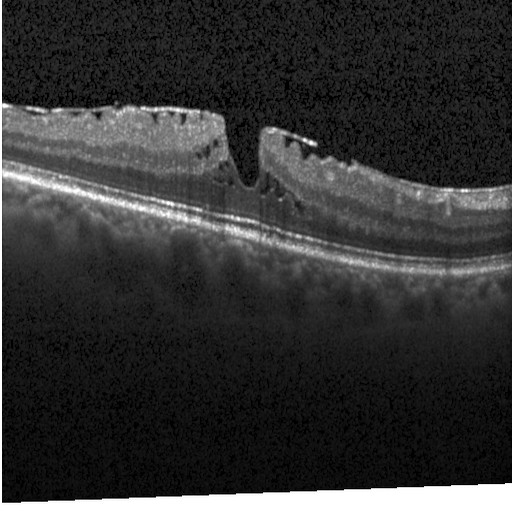
Retinal OCT B-scan. Diagnosis: diabetic macular edema (DME).